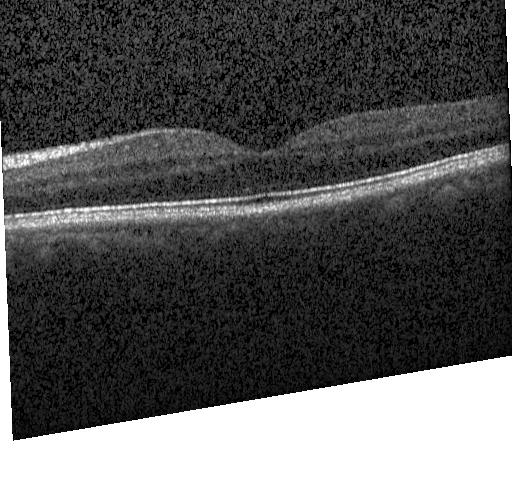

OCT finding: no choroidal neovascularization, no diabetic macular edema, and no drusen.